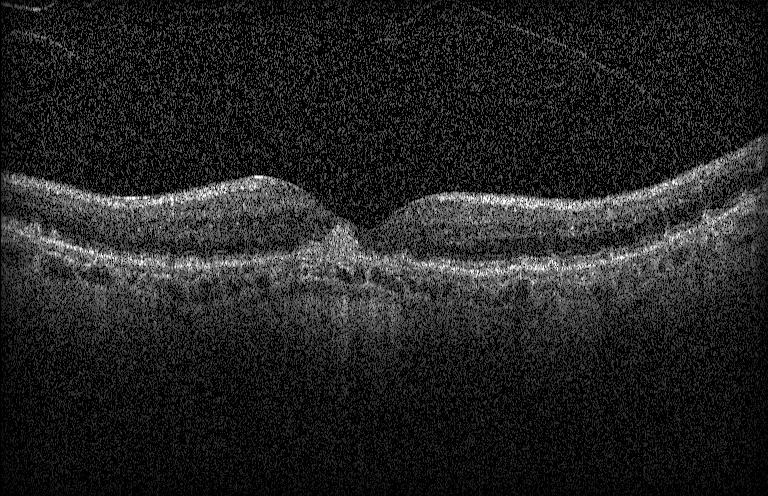

OCT scan showing CNV.